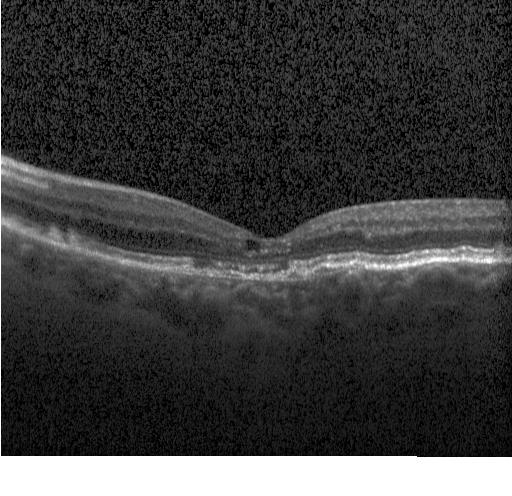
Heidelberg Spectralis. Horizontal scan through the fovea. Spectral-domain optical coherence tomography. OCT B-scan.
A choroidal neovascular membrane.